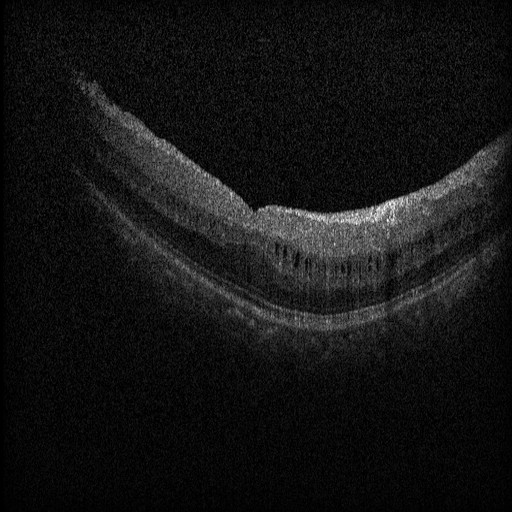
OCT B-scan · Heidelberg Spectralis · centered on the fovea · spectral-domain OCT — Finding: DME.